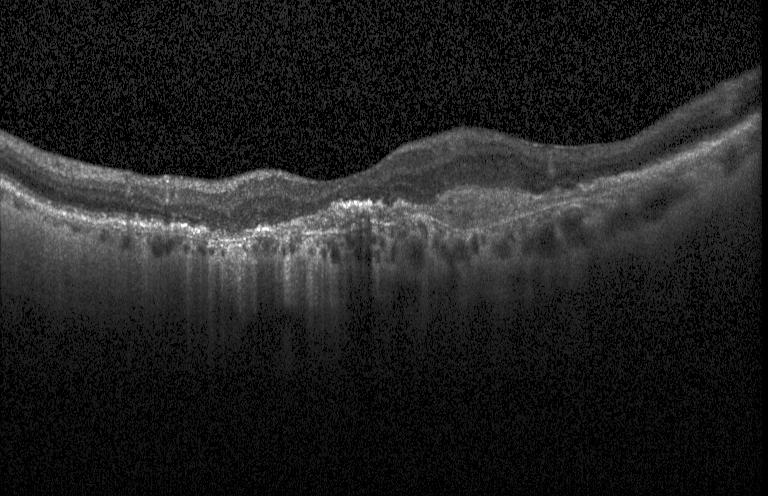 Optical coherence tomography scan. Diagnosis: a choroidal neovascular membrane.